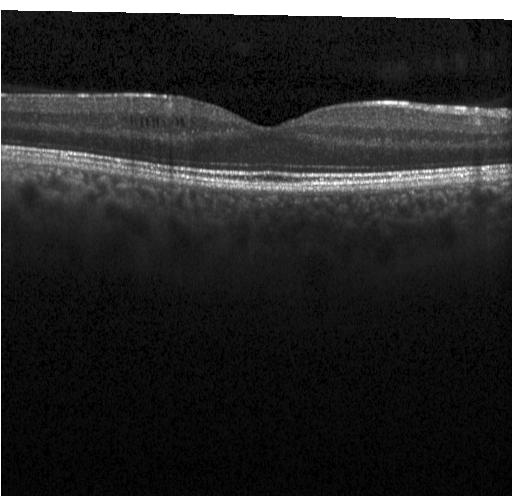

Horizontal scan through the fovea, Heidelberg Spectralis OCT system, spectral-domain optical coherence tomography, optical coherence tomography scan — Diagnosis: neither choroidal neovascularization, diabetic macular edema, nor drusen.